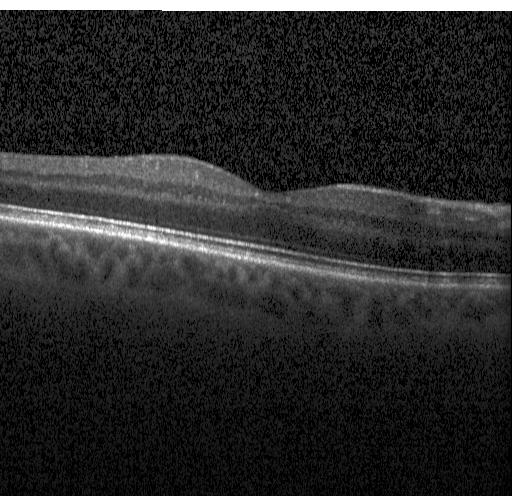

Optical coherence tomography scan. Centered on the fovea. Spectral-domain optical coherence tomography. Heidelberg Spectralis OCT system. Diagnosis: no choroidal neovascularization, diabetic macular edema, or drusen.